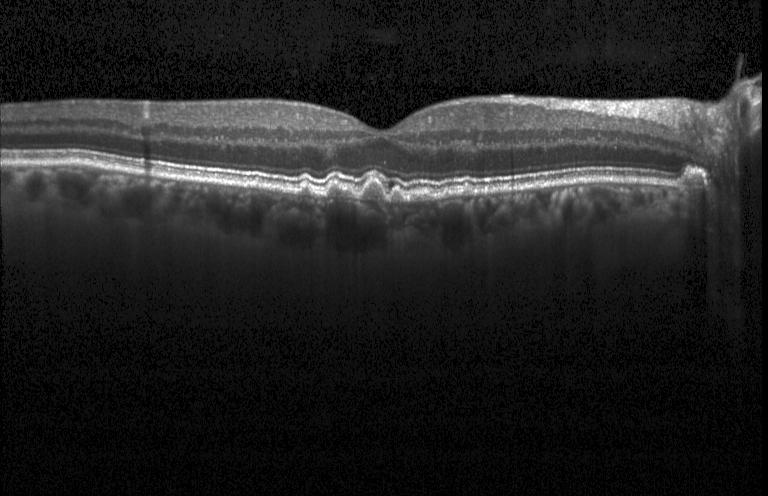

Macular scan · OCT line scan · SD-OCT · acquired on a Heidelberg Spectralis.
Diagnosis: drusen.